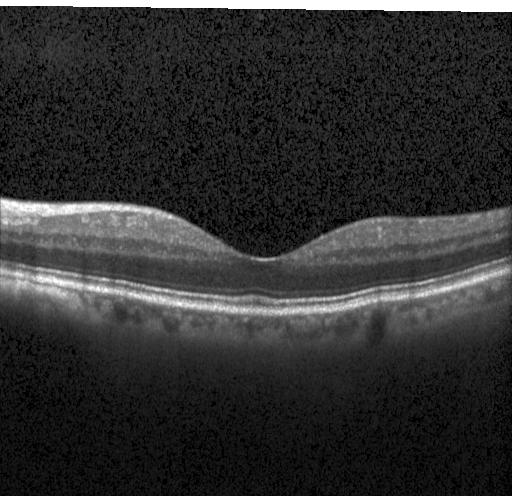
Retinal OCT cross-section · fovea-centered.
Diagnosis: neither choroidal neovascularization, diabetic macular edema, nor drusen.